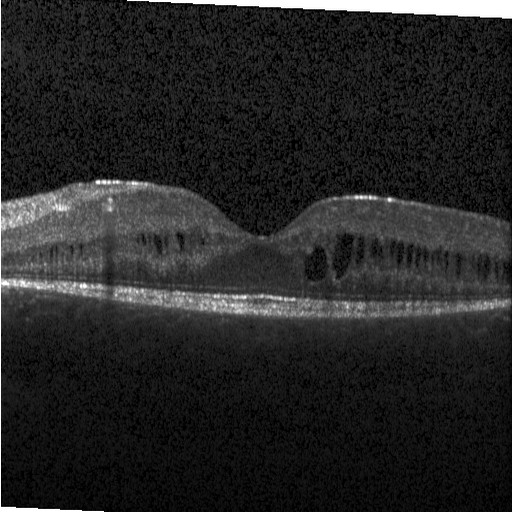

SD-OCT. Horizontal scan through the fovea. Retinal OCT cross-section
The scan shows DME.